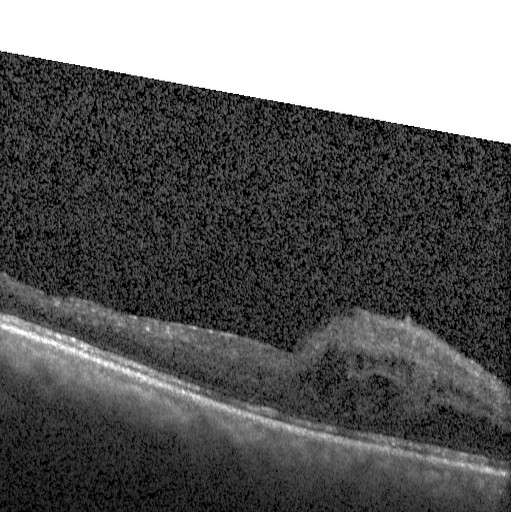

Retinal OCT cross-section. Fovea-centered. Acquired on a Heidelberg Spectralis — This B-scan demonstrates DME.